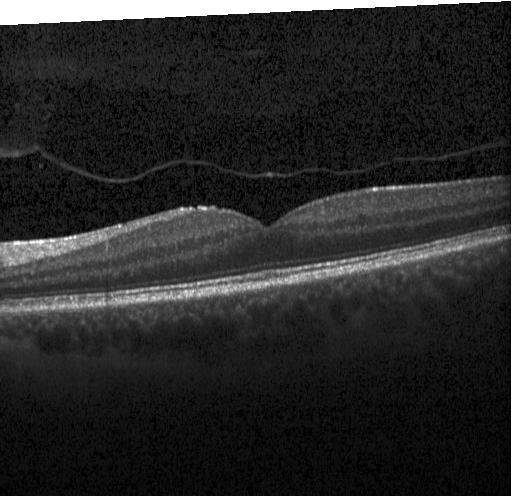 This B-scan demonstrates no evidence of choroidal neovascularization, diabetic macular edema, or drusen.